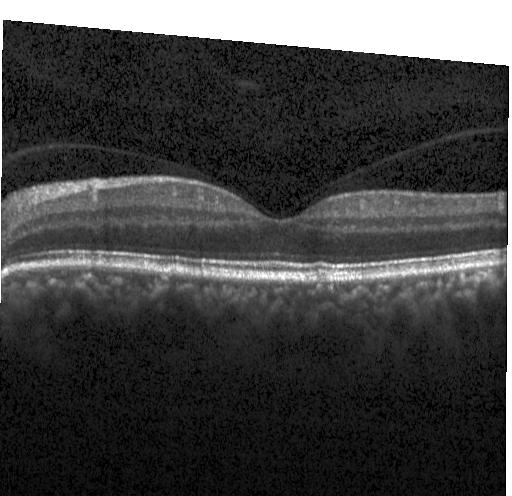
Impression: drusen.